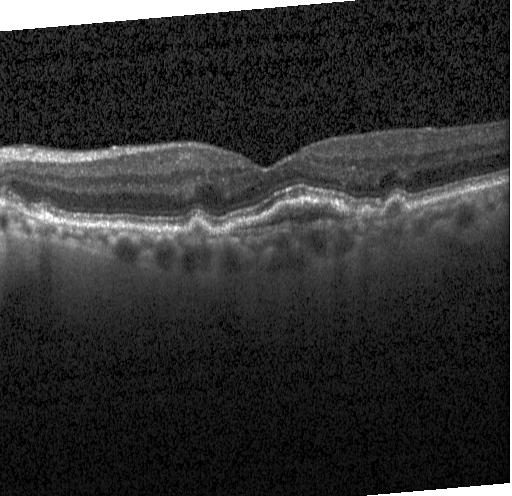

Finding: a choroidal neovascular membrane.